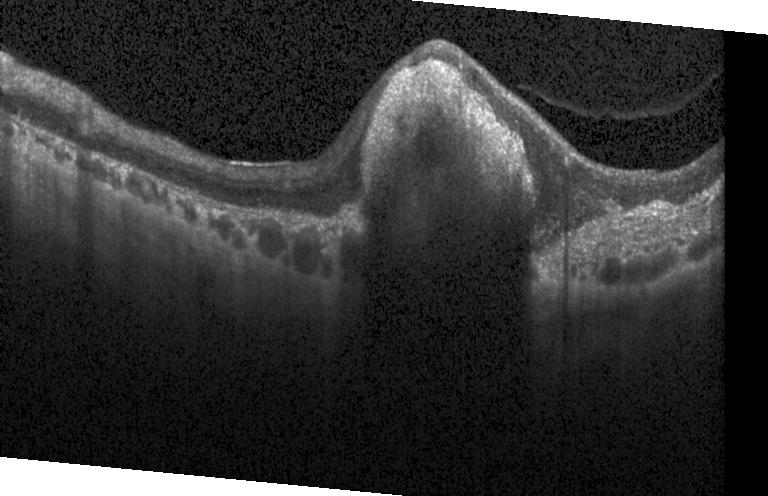 Macular scan · OCT B-scan · Heidelberg Spectralis · spectral-domain optical coherence tomography
Macular OCT: a choroidal neovascular membrane.